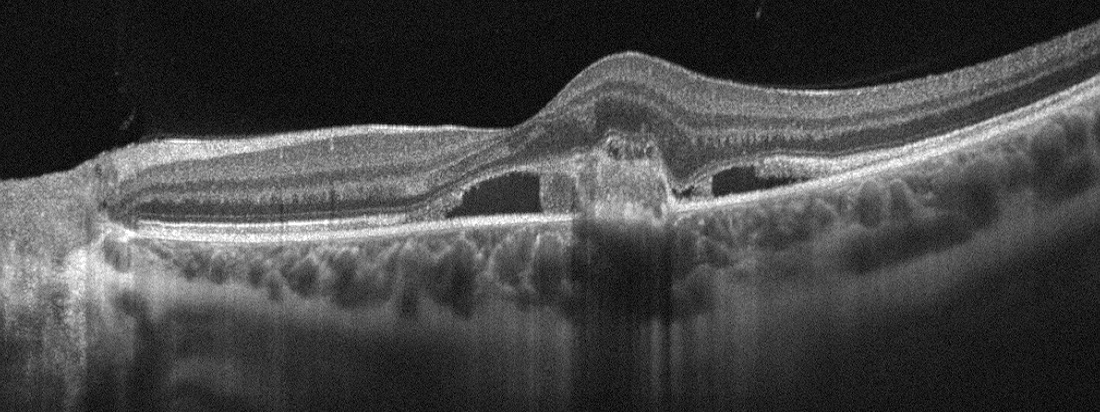 Optical coherence tomography B-scan. Fovea-centered. Finding: age-related macular degeneration (AMD).